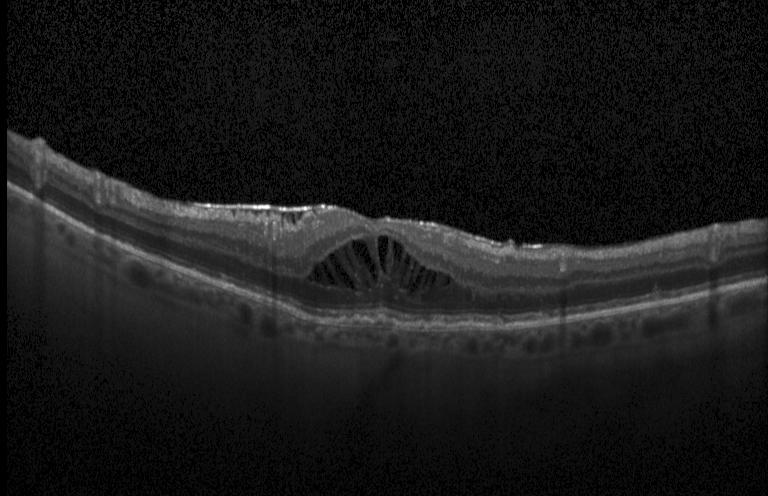
Spectral-domain optical coherence tomography. Optical coherence tomography B-scan
Finding: diabetic macular edema.